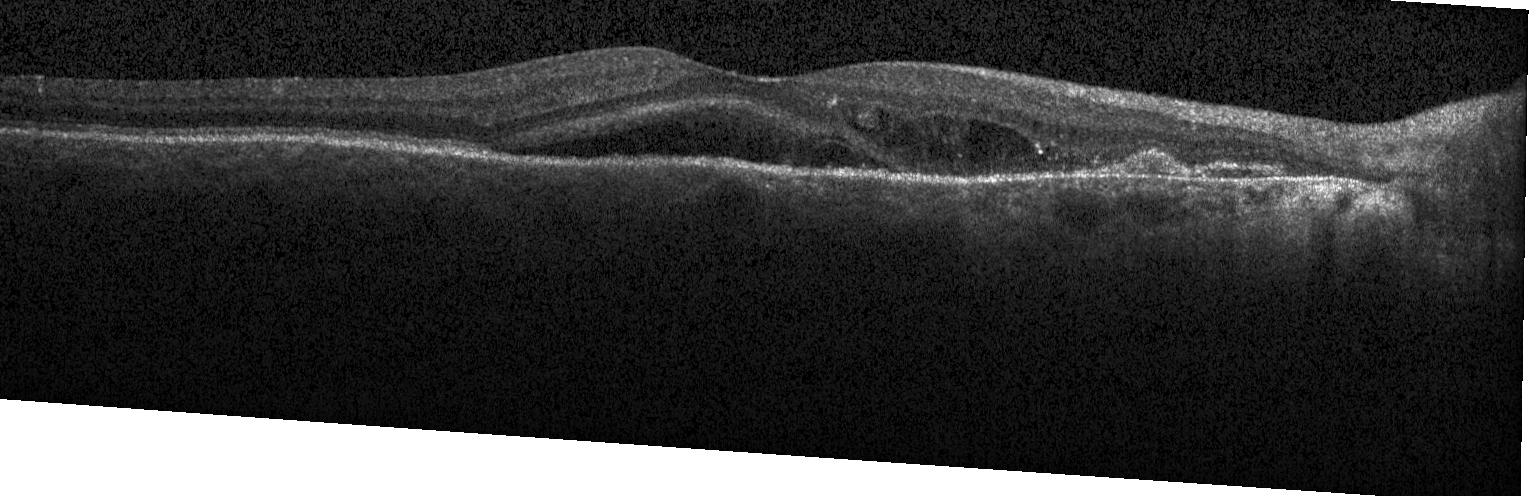
OCT line scan.
Finding: a choroidal neovascular membrane.